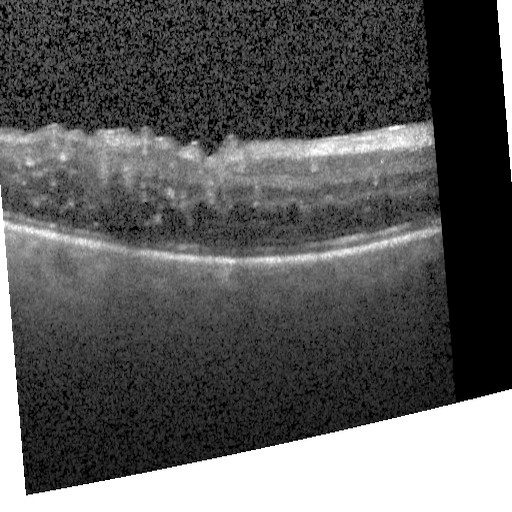
OCT line scan. Spectral-domain OCT. Horizontal scan through the fovea — Dx: DME.